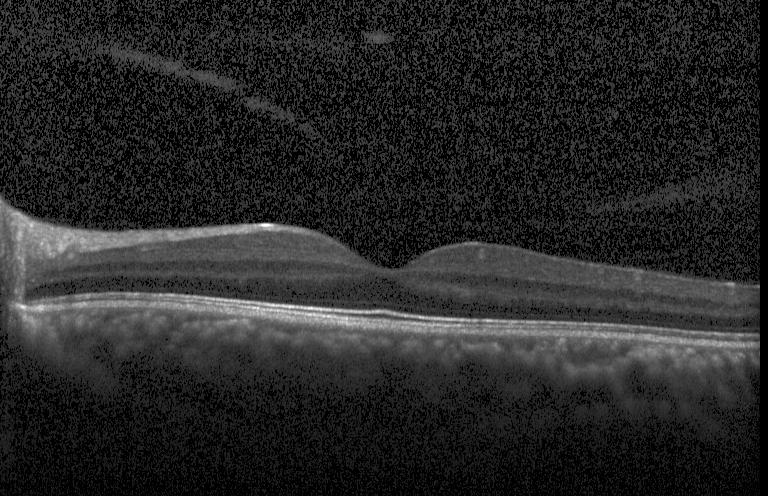
Retinal OCT B-scan, acquired on a Heidelberg Spectralis — This B-scan demonstrates neither choroidal neovascularization, diabetic macular edema, nor drusen.